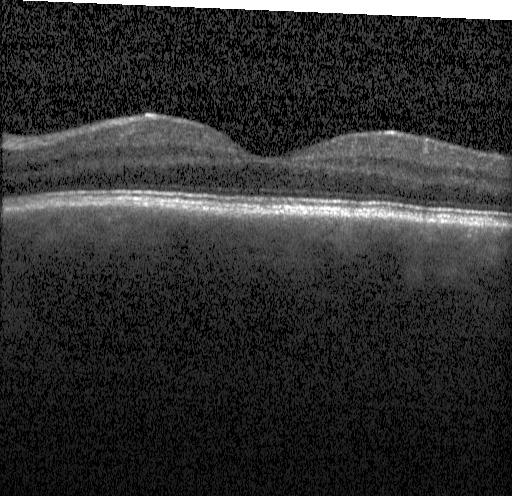 Retinal OCT cross-section. Fovea-centered — Diagnosis: no evidence of choroidal neovascularization, diabetic macular edema, or drusen.